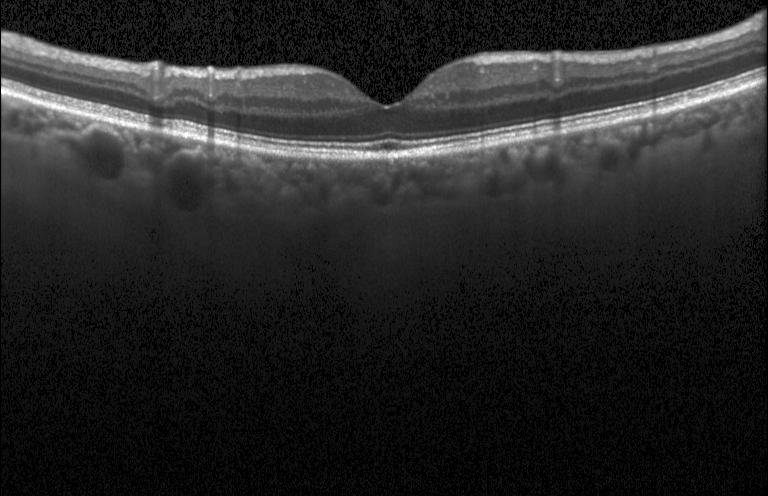
OCT B-scan showing neither CNV, DME, nor drusen.